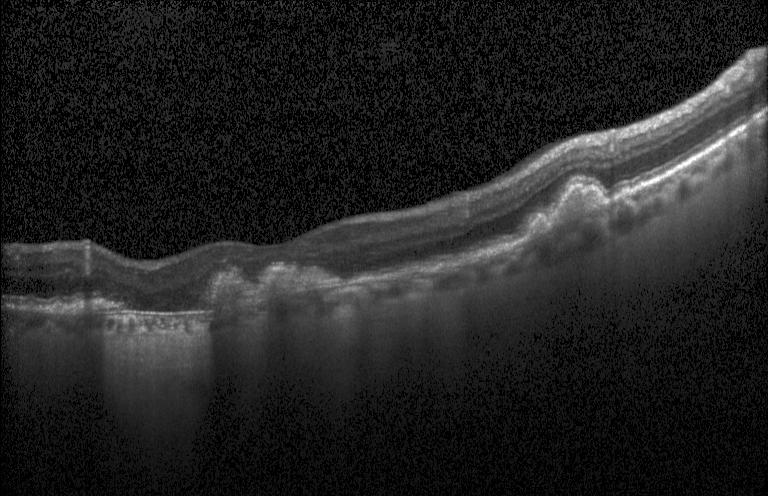
Choroidal neovascularization.